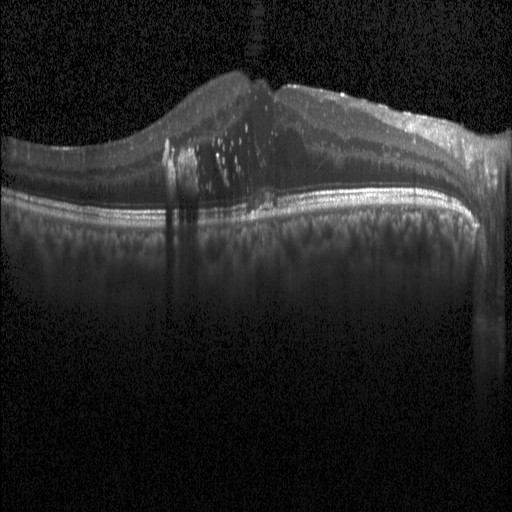 Diagnosis: diabetic macular edema.